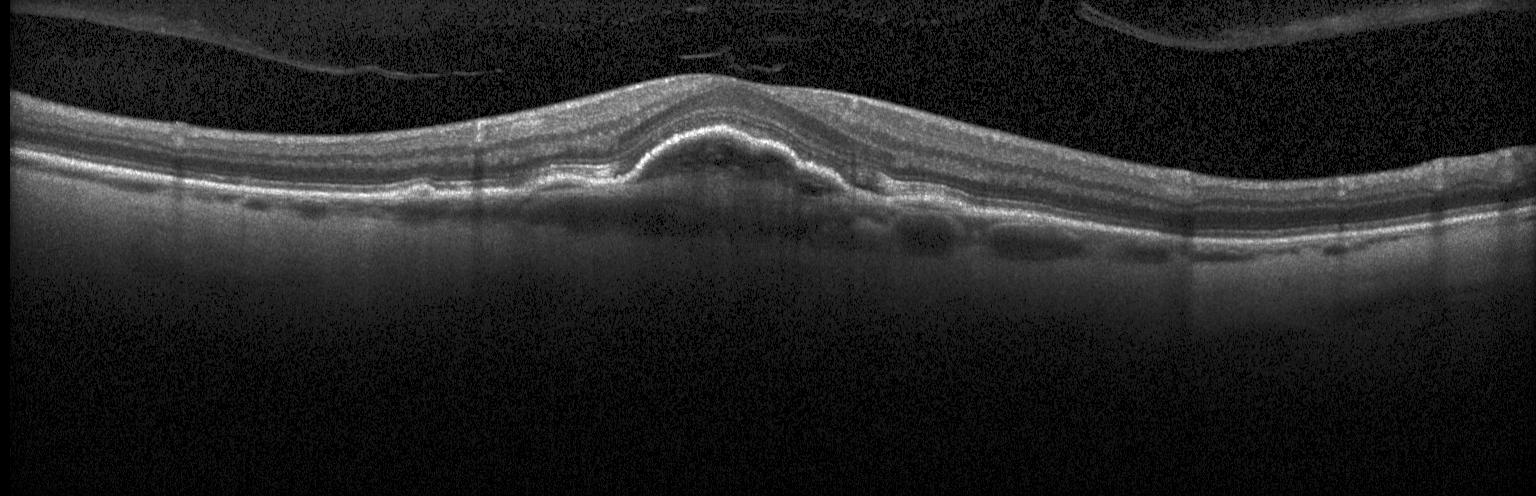
Spectral-domain OCT, OCT B-scan, Heidelberg Spectralis, fovea-centered.
Impression: a choroidal neovascular membrane.